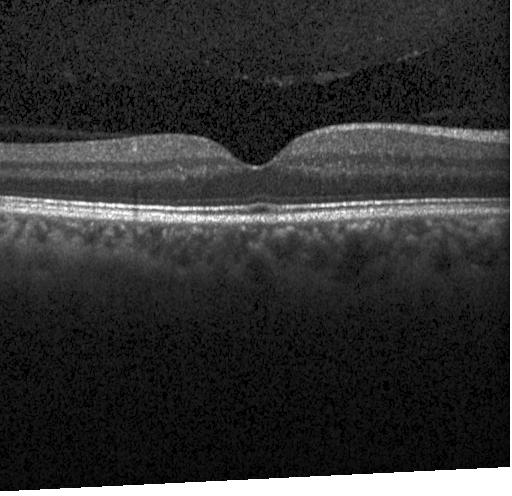
Through the macula, optical coherence tomography scan, SD-OCT
The scan shows no choroidal neovascularization, diabetic macular edema, or drusen.